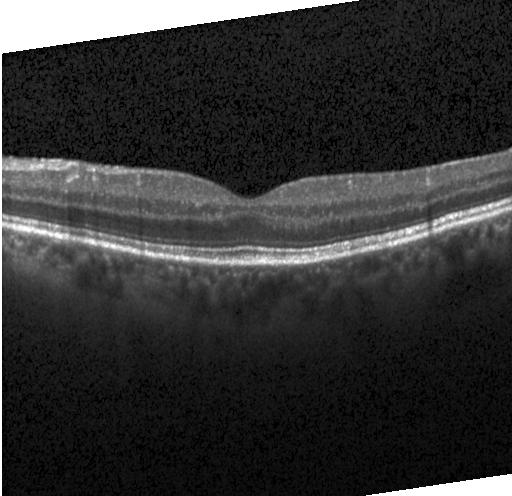 Retinal OCT cross-section. Instrument: Heidelberg Spectralis. SD-OCT.
Assessment: no CNV, DME, or drusen.